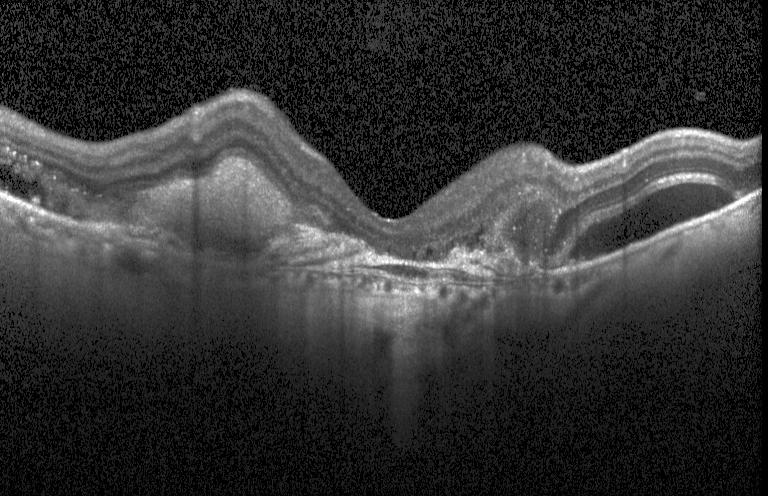 Spectral-domain OCT B-scan: CNV.